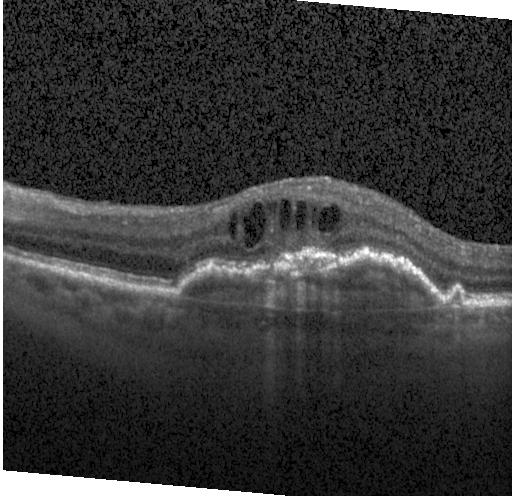
Instrument: Heidelberg Spectralis; retinal OCT cross-section; SD-OCT; macular scan
Assessment: CNV.